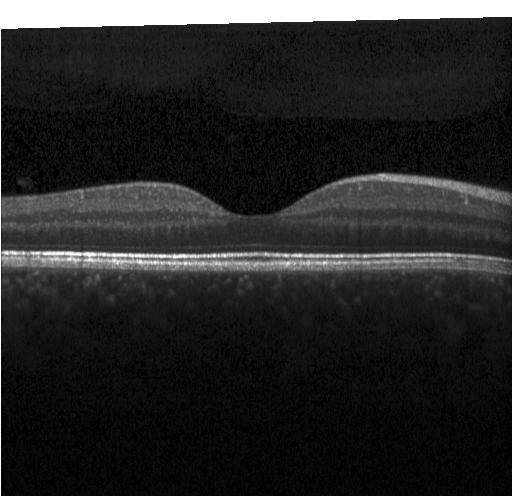

Fovea-centered, SD-OCT, OCT line scan, Heidelberg Spectralis OCT system — Dx: no choroidal neovascularization, diabetic macular edema, or drusen.